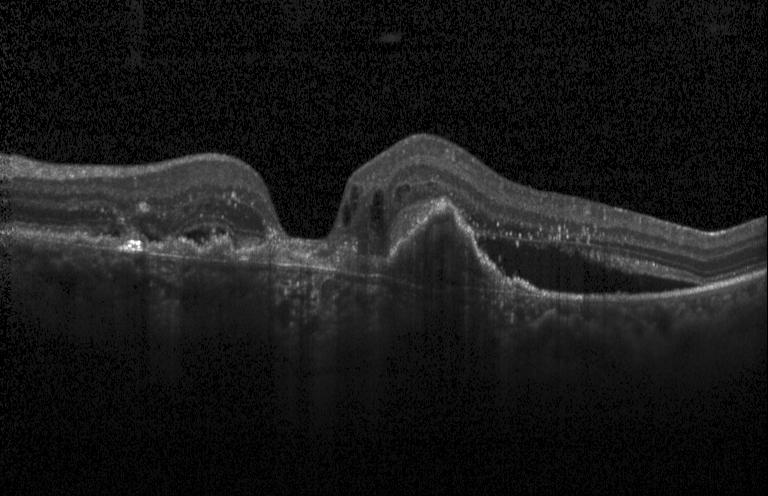

Macular OCT demonstrating a choroidal neovascular membrane.